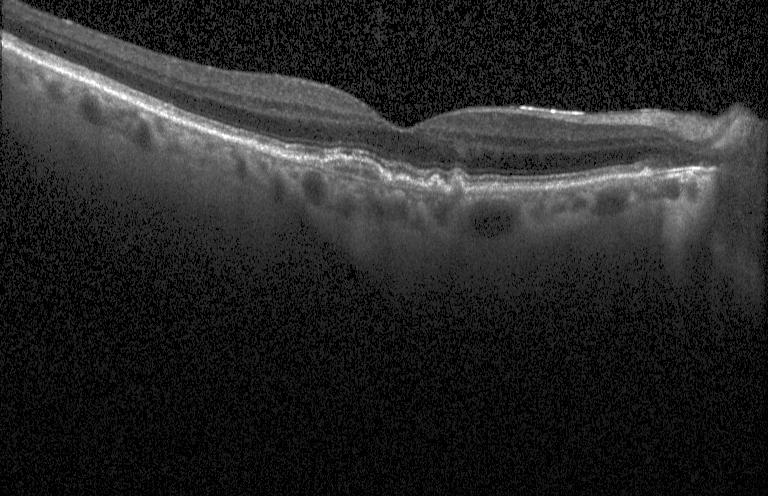
Retinal OCT cross-section. Diagnosis: a choroidal neovascular membrane.